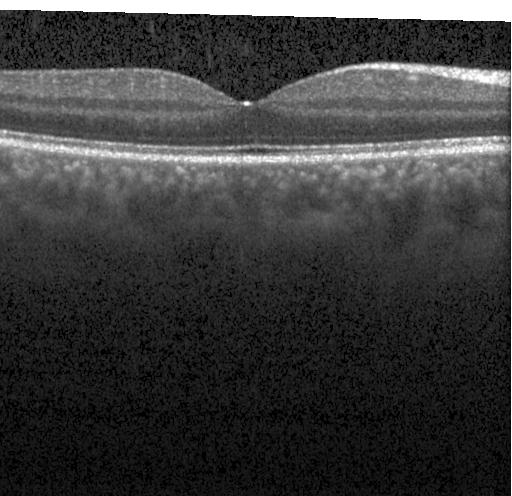
OCT B-scan showing no choroidal neovascularization, diabetic macular edema, or drusen.